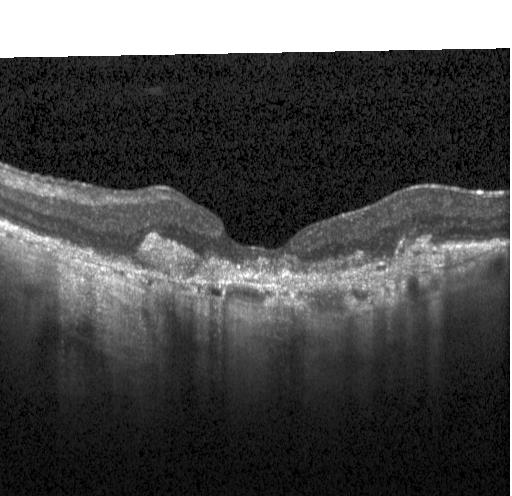 Dx: CNV.